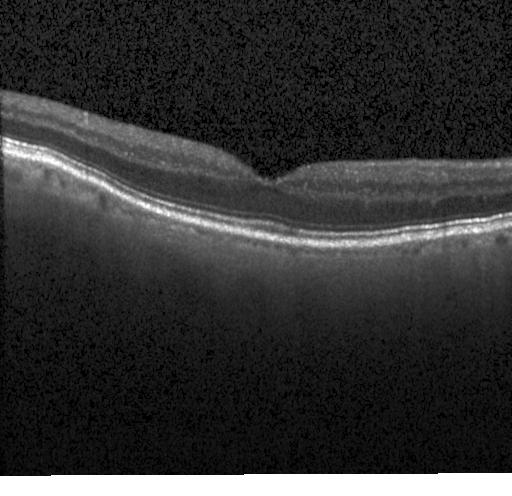 Optical coherence tomography B-scan; macular scan — Diagnosis: no choroidal neovascularization, no diabetic macular edema, and no drusen.